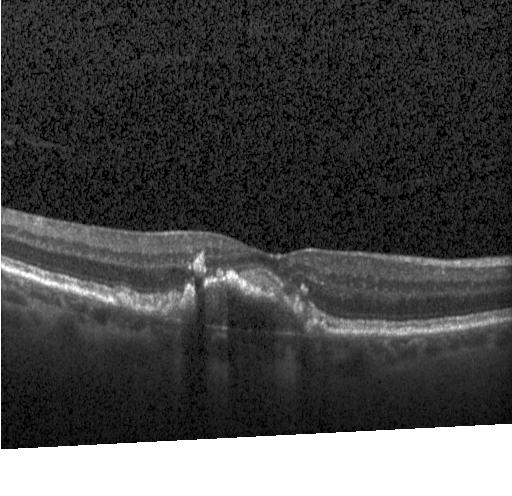 OCT B-scan
Macular OCT: CNV.